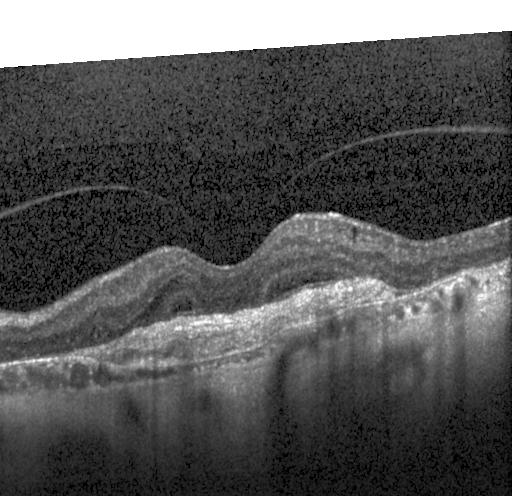

Spectral-domain optical coherence tomography · Heidelberg Spectralis OCT system · OCT B-scan · centered on the fovea — OCT finding: choroidal neovascularization (CNV).